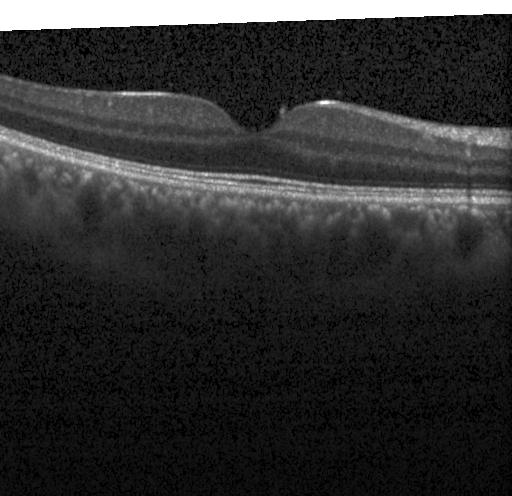
Impression: no choroidal neovascularization, diabetic macular edema, or drusen.